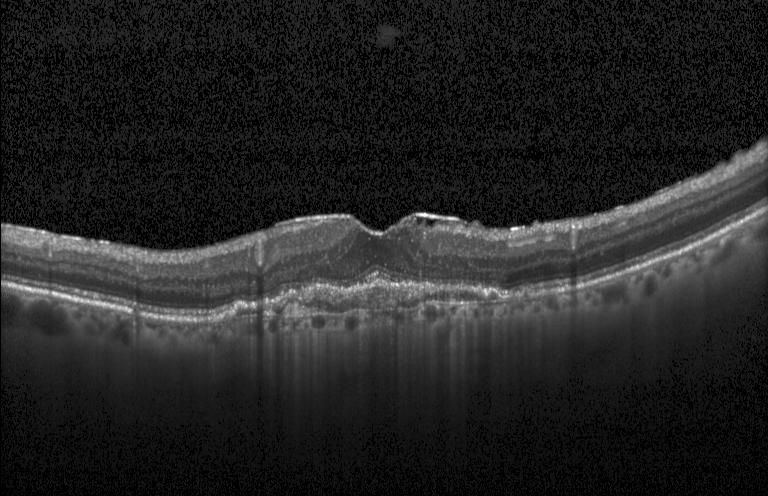

Retinal OCT B-scan, acquired on a Heidelberg Spectralis
Diagnosis: choroidal neovascularization.